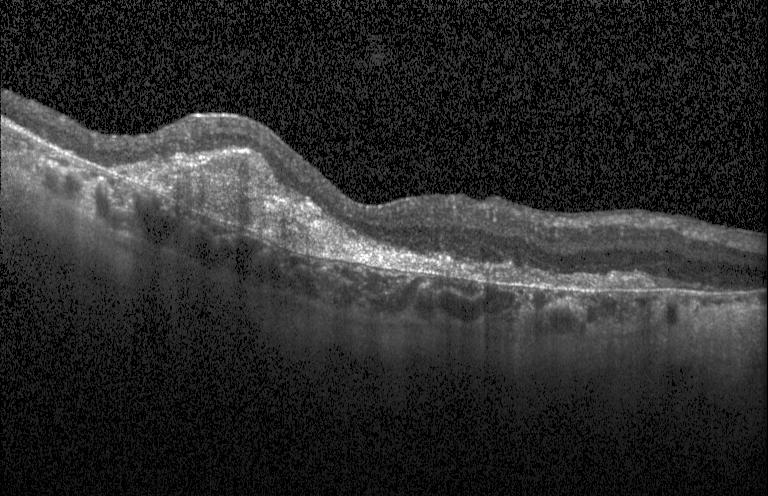
Spectral-domain optical coherence tomography, instrument: Heidelberg Spectralis, optical coherence tomography B-scan. This B-scan demonstrates choroidal neovascularization.